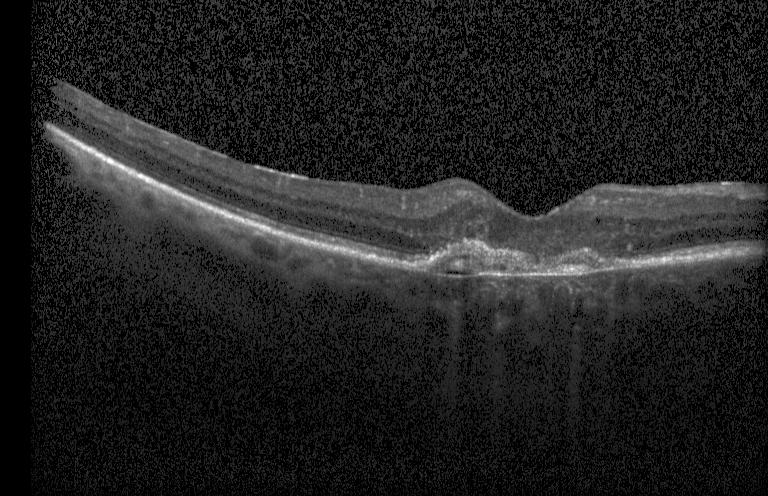
Diagnosis: a choroidal neovascular membrane.